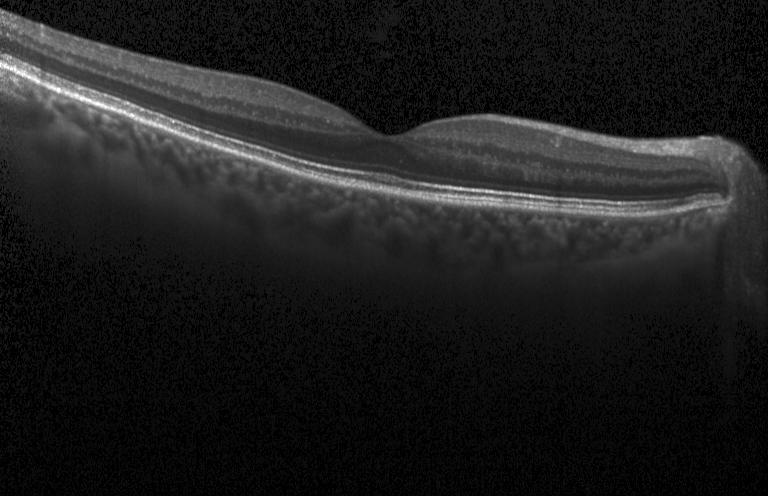

Optical coherence tomography scan
Finding: no CNV, no DME, and no drusen.